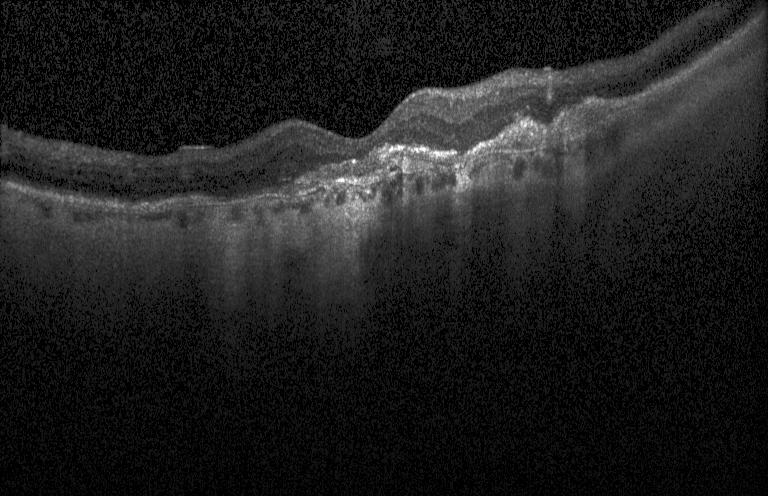

Heidelberg Spectralis OCT system; optical coherence tomography scan; SD-OCT. The scan shows a choroidal neovascular membrane.